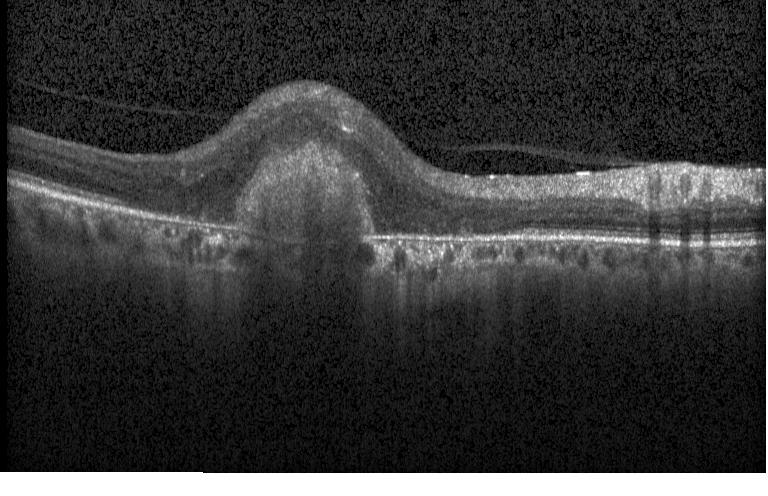

Optical coherence tomography scan. Instrument: Heidelberg Spectralis
Impression: choroidal neovascularization.